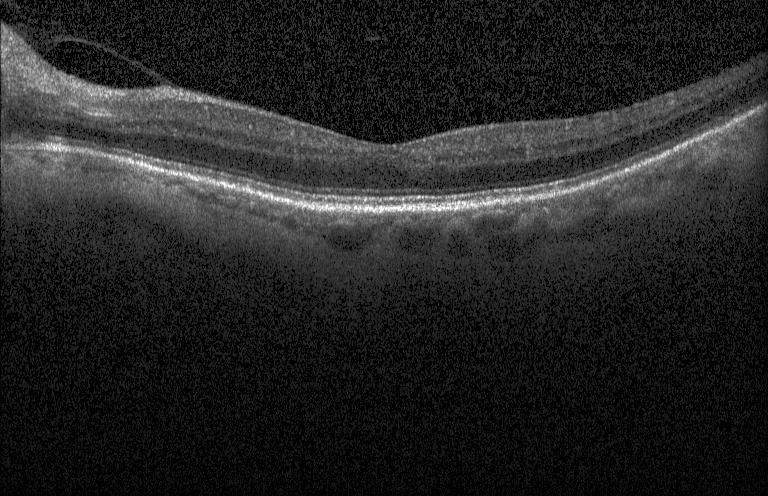
Finding: no choroidal neovascularization, no diabetic macular edema, and no drusen.